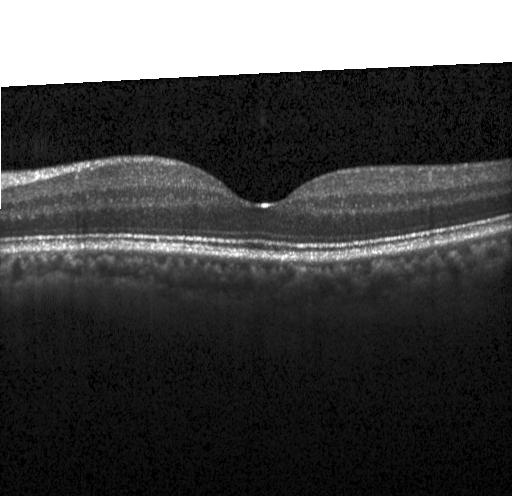

Impression: no choroidal neovascularization, no diabetic macular edema, and no drusen.